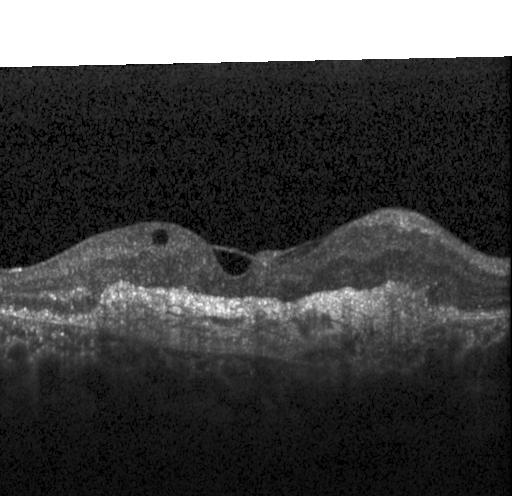
Optical coherence tomography scan.
The scan shows choroidal neovascularization (CNV).